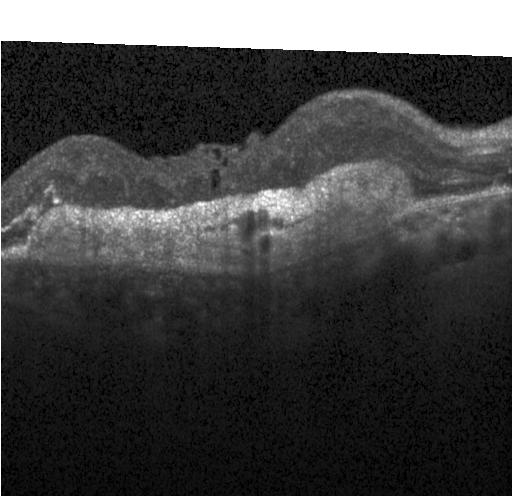
Retinal OCT B-scan. SD-OCT.
Dx: a choroidal neovascular membrane.